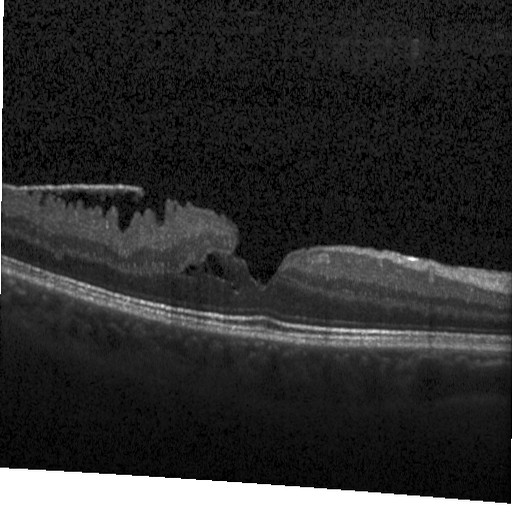

OCT line scan; instrument: Heidelberg Spectralis; macular scan; spectral-domain OCT
Impression: DME.